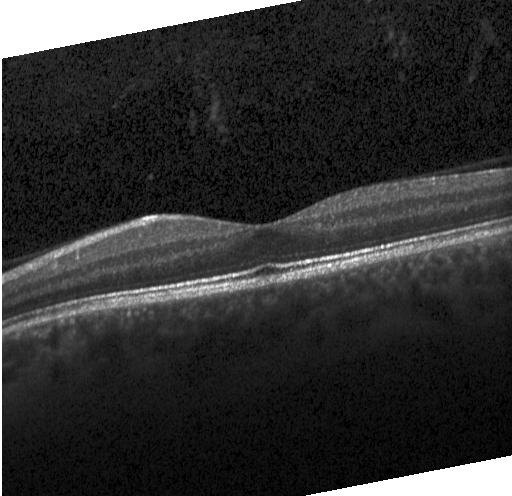
Spectral-domain optical coherence tomography · OCT B-scan · fovea-centered
The scan shows no choroidal neovascularization, diabetic macular edema, or drusen.